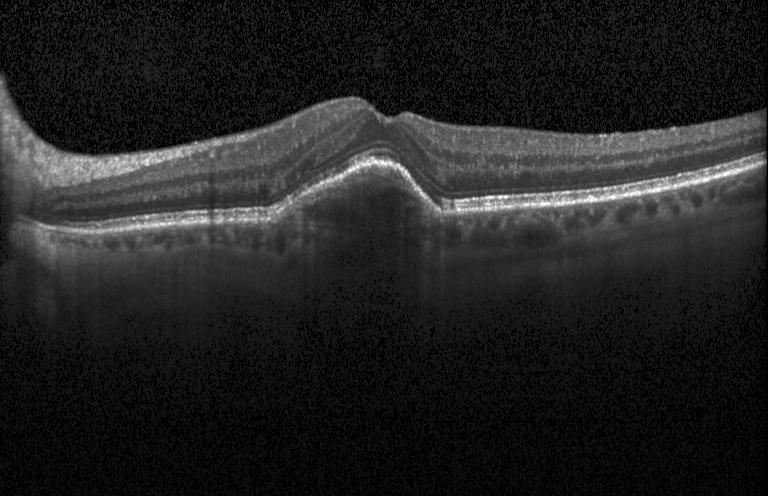
OCT B-scan
Impression: choroidal neovascularization (CNV).